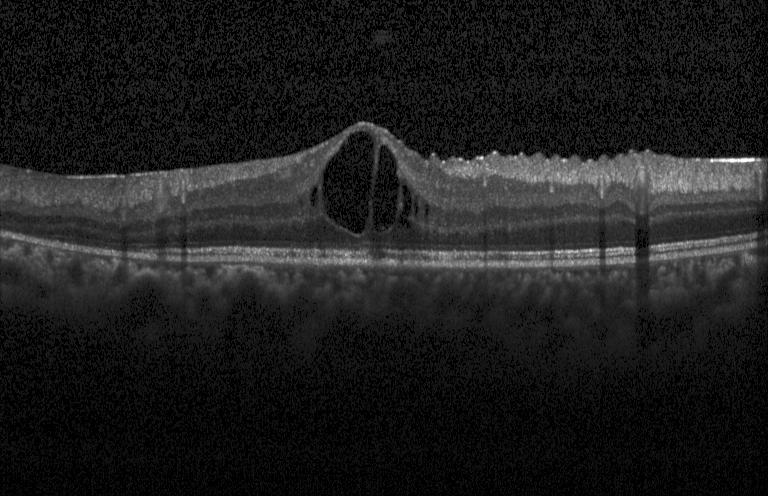

Retinal OCT B-scan, macular scan — Diagnosis: DME.